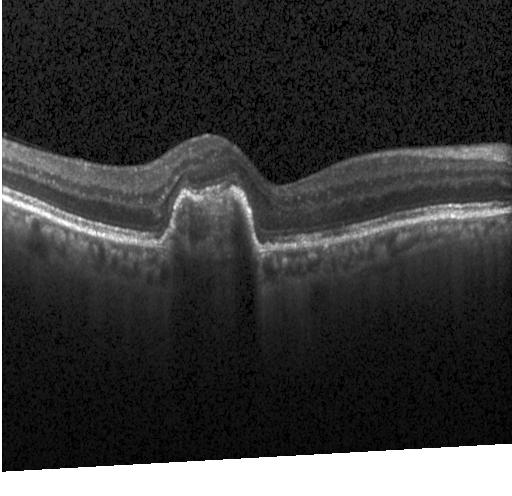 Horizontal scan through the fovea · OCT B-scan
Impression: CNV.